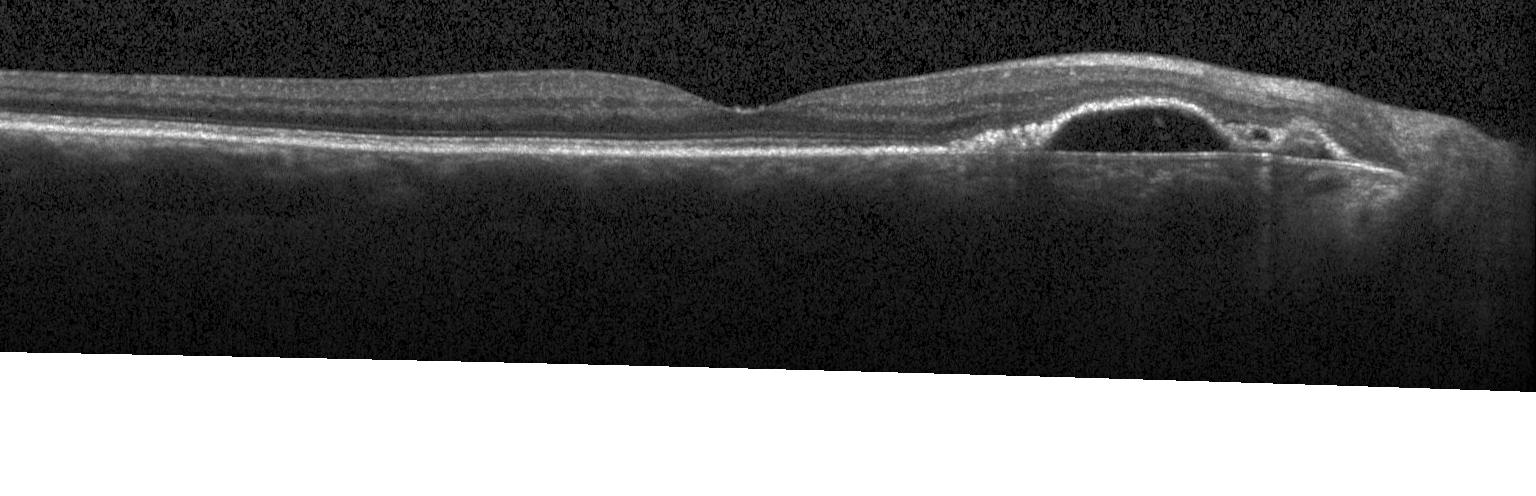

Dx: choroidal neovascularization (CNV).